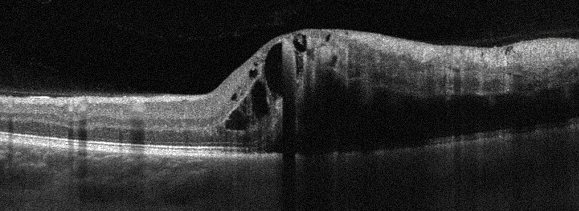 Left eye, retinal OCT cross-section.
The scan shows retinal vein occlusion.